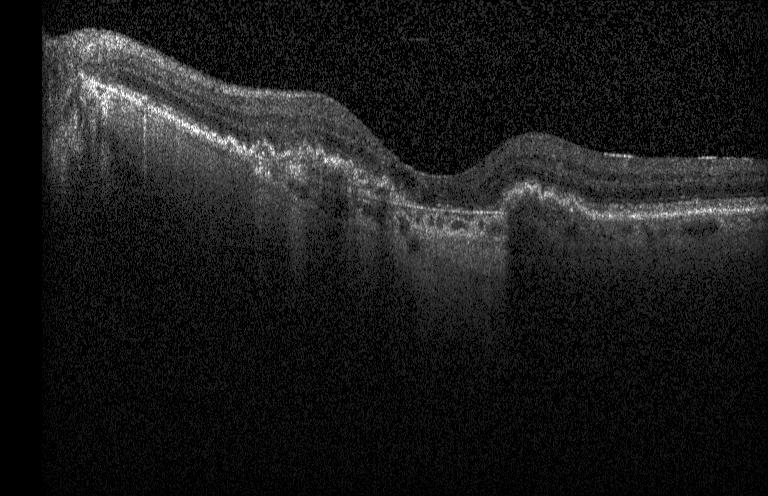
CNV.